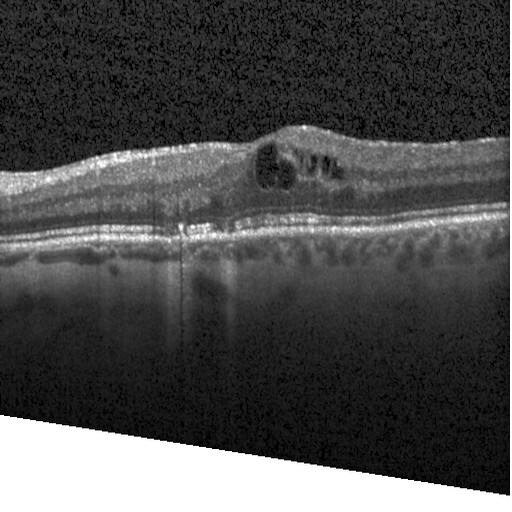

Optical coherence tomography B-scan · spectral-domain optical coherence tomography
Diagnosis: diabetic macular edema (DME).